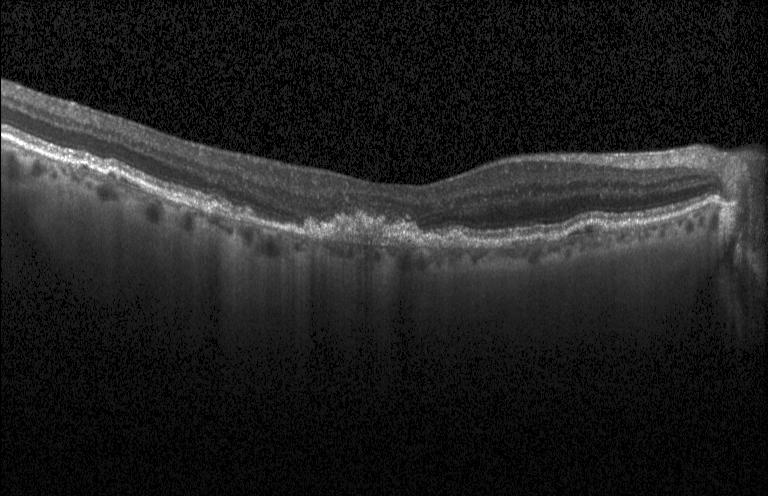
Optical coherence tomography scan; fovea-centered; instrument: Heidelberg Spectralis; spectral-domain OCT. Macular OCT: CNV.